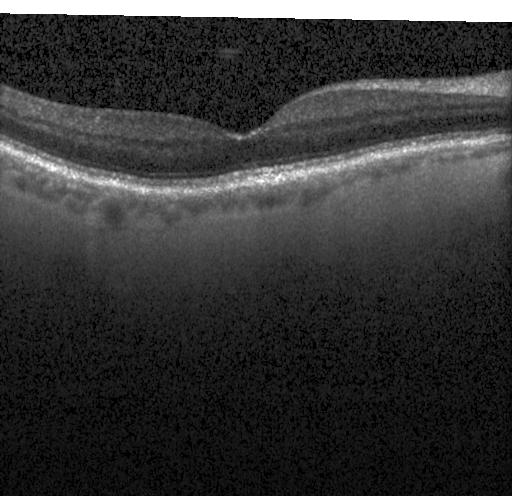 Centered on the fovea · OCT line scan — Impression: no evidence of choroidal neovascularization, diabetic macular edema, or drusen.